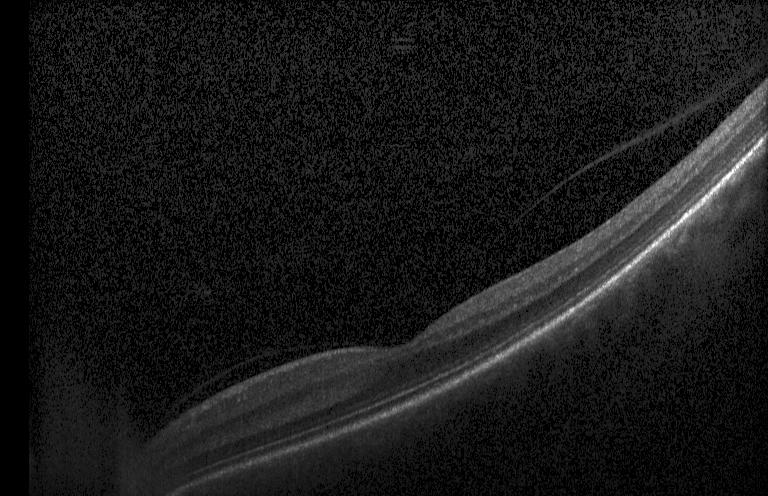 Optical coherence tomography B-scan.
Impression: no choroidal neovascularization, no diabetic macular edema, and no drusen.